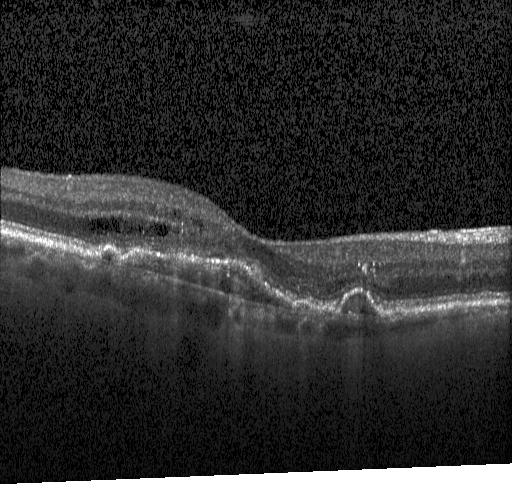 Impression: choroidal neovascularization (CNV).